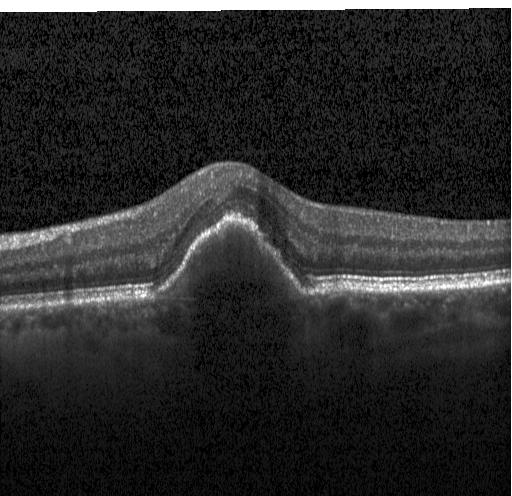
Retinal OCT B-scan · fovea-centered
Diagnosis: a choroidal neovascular membrane.